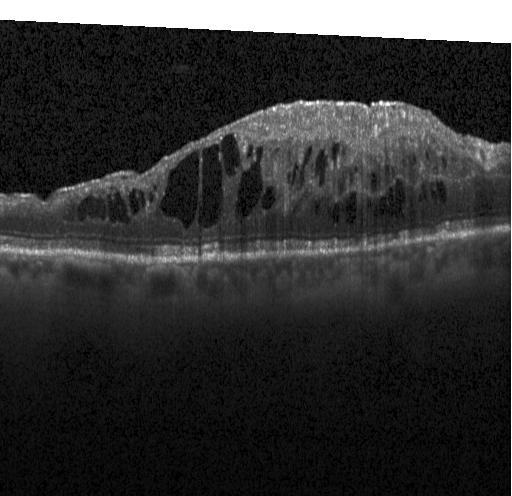 Impression: diabetic macular edema.